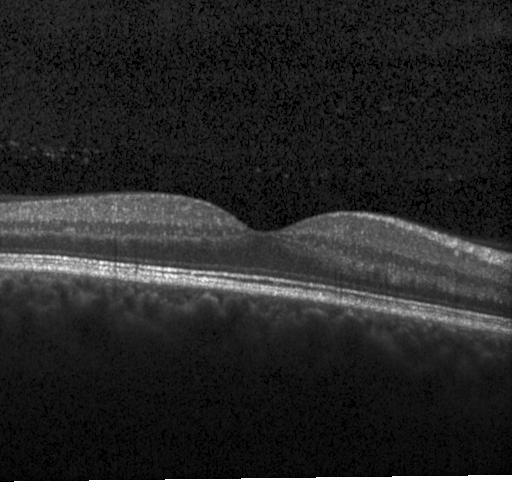 OCT B-scan
Neither choroidal neovascularization, diabetic macular edema, nor drusen.